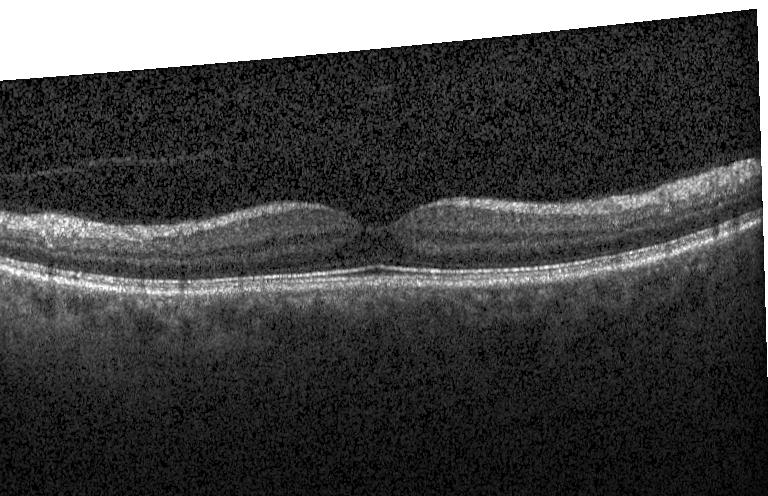 Macular scan; spectral-domain OCT; retinal OCT B-scan; instrument: Heidelberg Spectralis.
No CNV, no DME, and no drusen.